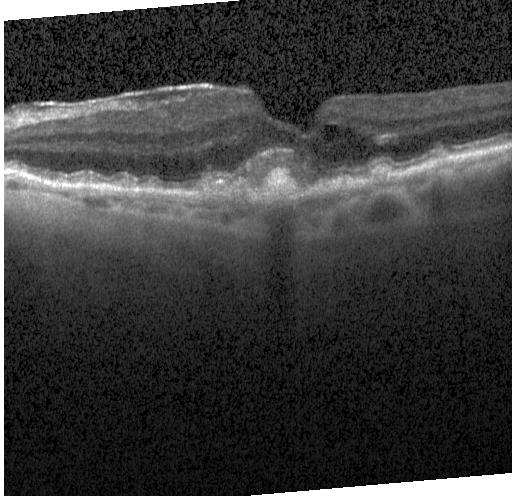
Heidelberg Spectralis · SD-OCT · OCT B-scan
Impression: choroidal neovascularization (CNV).